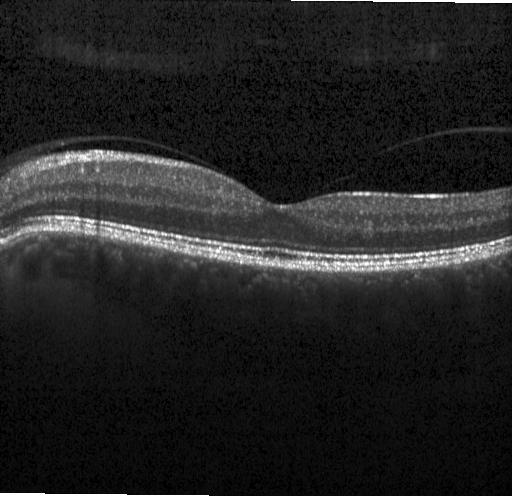
Diagnosis: no choroidal neovascularization, diabetic macular edema, or drusen.